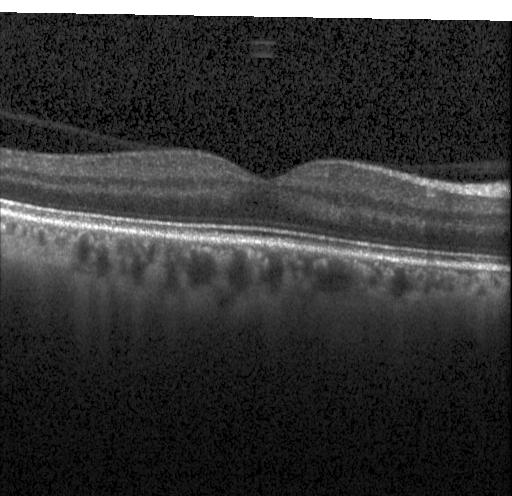
OCT scan showing no evidence of CNV, DME, or drusen.